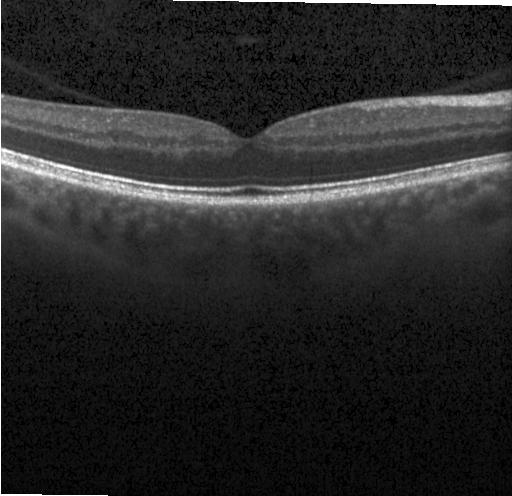
Macular OCT: no choroidal neovascularization, diabetic macular edema, or drusen.